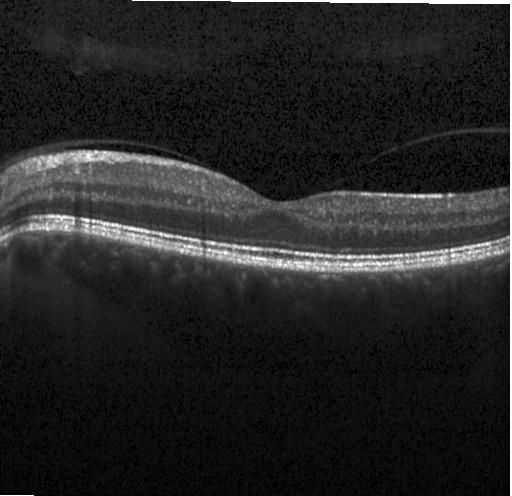
Macular scan. Optical coherence tomography B-scan. Heidelberg Spectralis.
The scan shows no choroidal neovascularization, diabetic macular edema, or drusen.